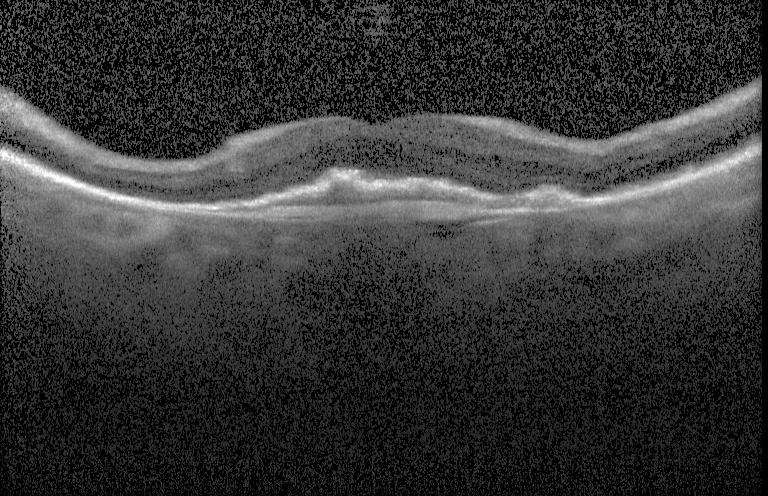
Macular OCT: a choroidal neovascular membrane.